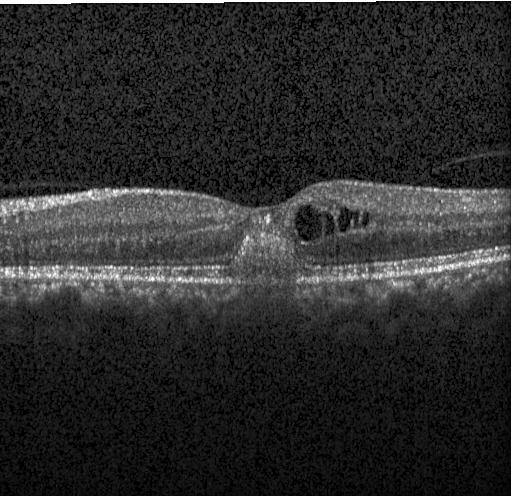
Finding: a choroidal neovascular membrane.